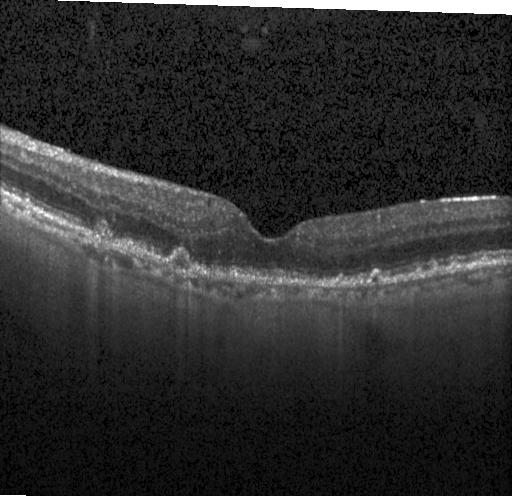

Retinal OCT cross-section · spectral-domain optical coherence tomography · horizontal scan through the fovea · Heidelberg Spectralis OCT system
Impression: CNV.